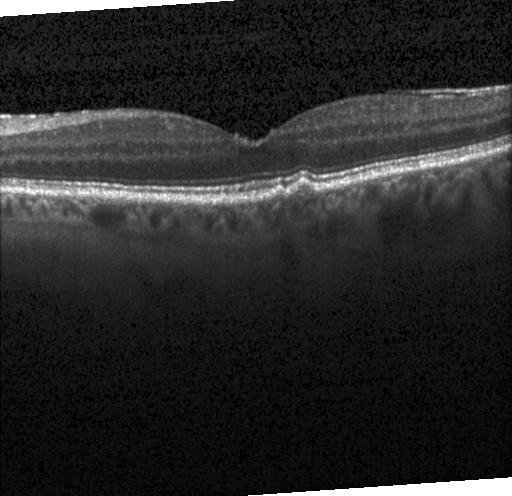
Acquired on a Heidelberg Spectralis; OCT line scan; through the macula; SD-OCT. Dx: sub-RPE drusenoid deposits.